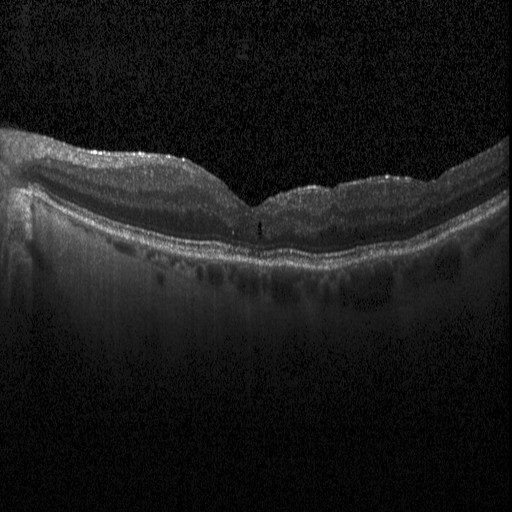
Instrument: Heidelberg Spectralis, optical coherence tomography scan
Finding: diabetic macular edema (DME).